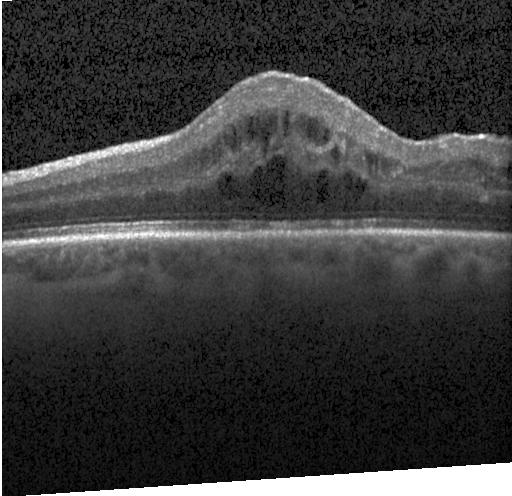

Spectral-domain optical coherence tomography, retinal OCT B-scan. Dx: DME.